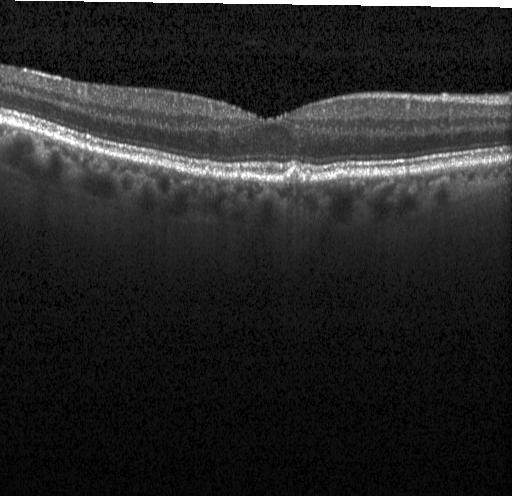 Acquired on a Heidelberg Spectralis. Optical coherence tomography scan
Diagnosis: multiple drusen.